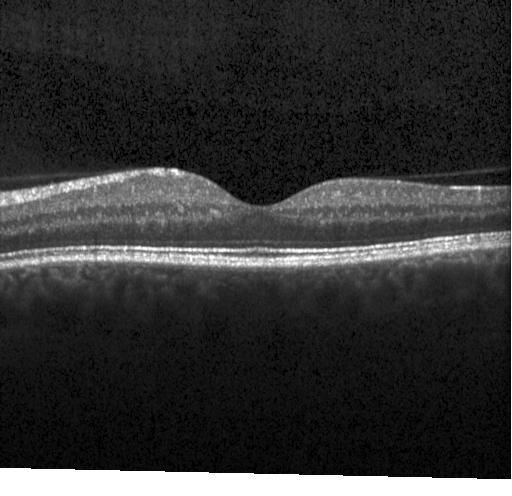 Horizontal scan through the fovea · Heidelberg Spectralis · spectral-domain optical coherence tomography · optical coherence tomography scan. Assessment: no CNV, no DME, and no drusen.